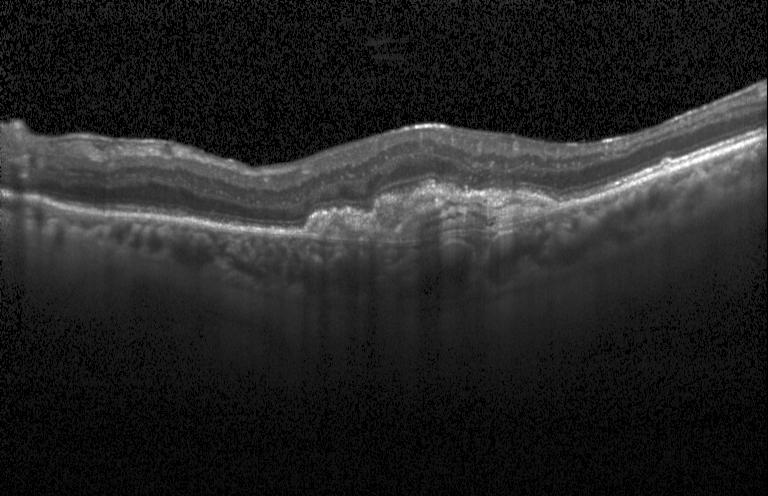

Optical coherence tomography scan.
Impression: CNV.